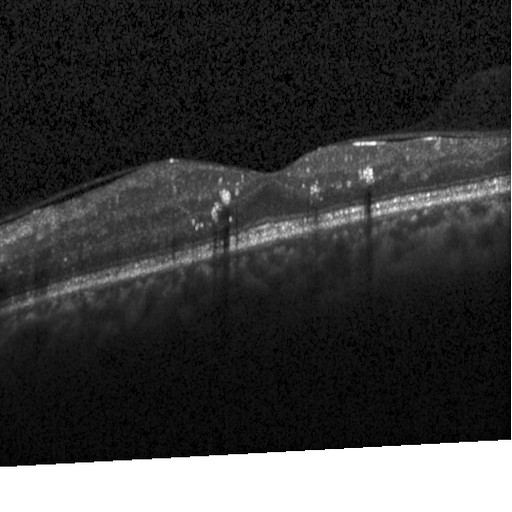
OCT finding: DME.